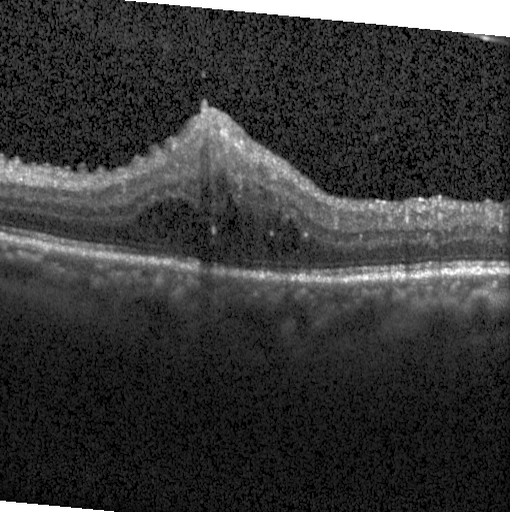
Dx: diabetic macular edema (DME).